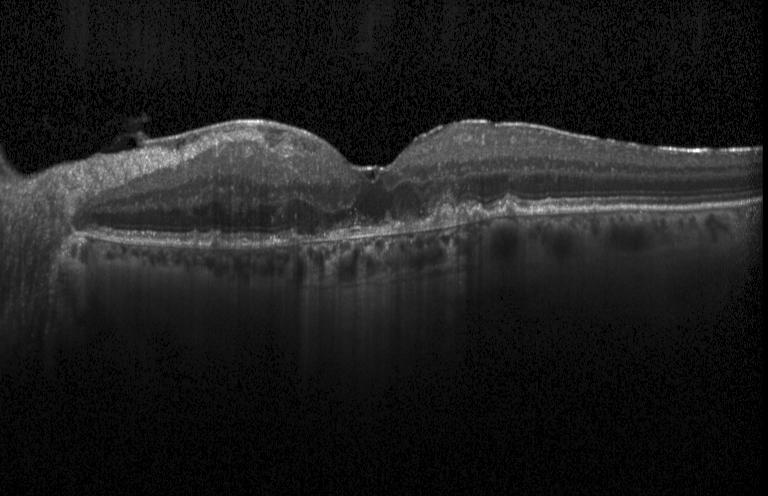
Dx: a choroidal neovascular membrane.